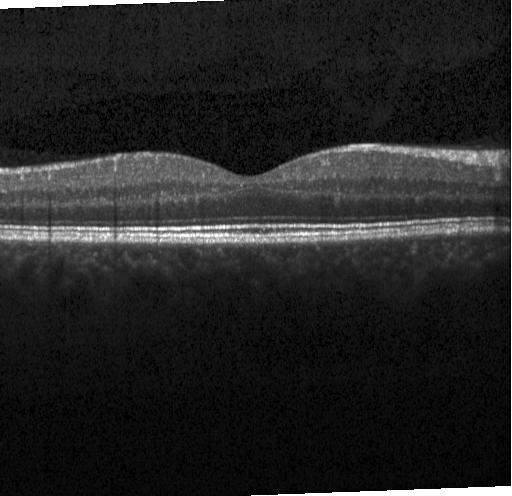 SD-OCT, horizontal scan through the fovea, Heidelberg Spectralis, OCT line scan.
This B-scan demonstrates no choroidal neovascularization, no diabetic macular edema, and no drusen.